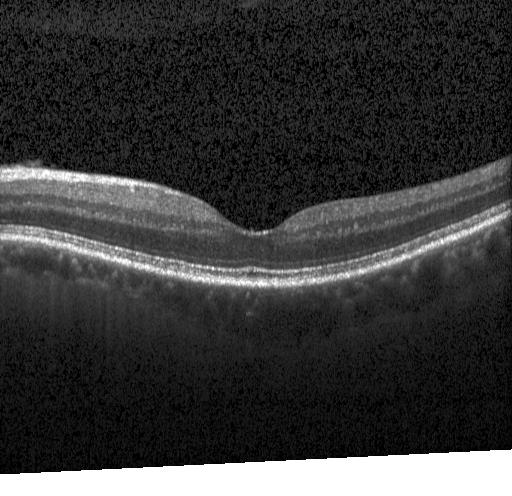

Macular OCT demonstrating no CNV, no DME, and no drusen.